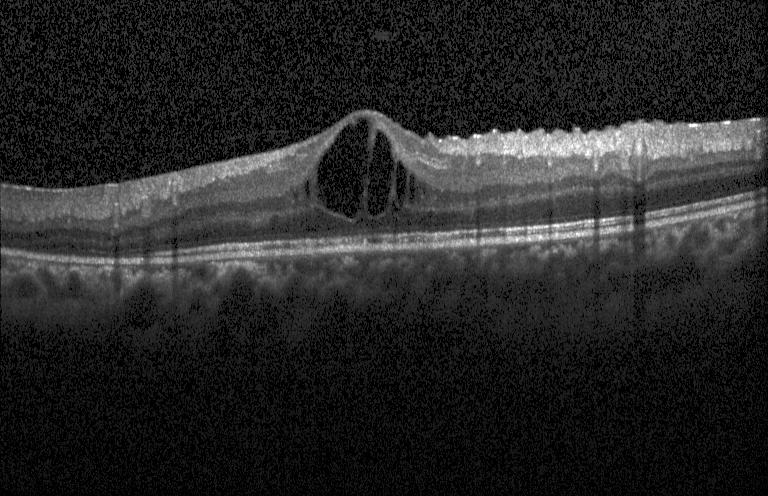 OCT line scan.
The scan shows diabetic macular edema.